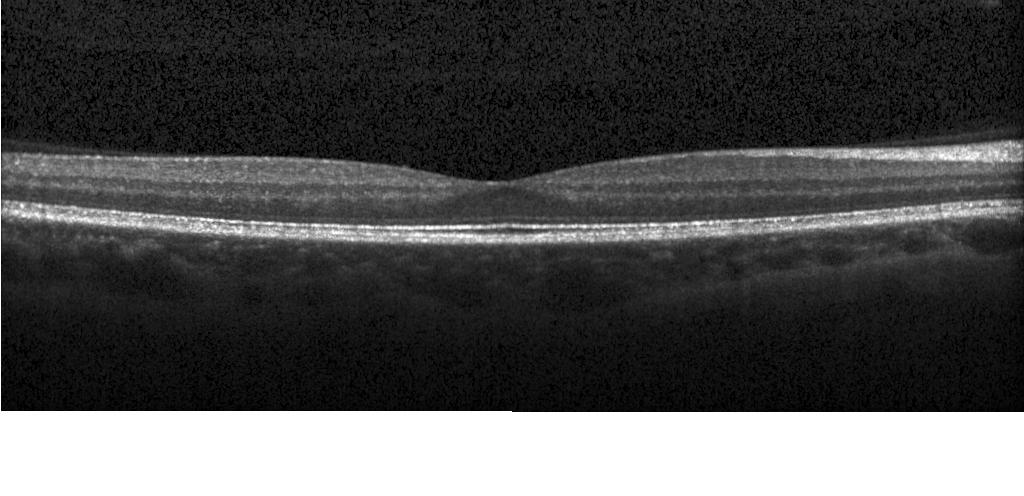

Spectral-domain OCT. Heidelberg Spectralis OCT system. OCT line scan. Macular scan.
Finding: no choroidal neovascularization, no diabetic macular edema, and no drusen.